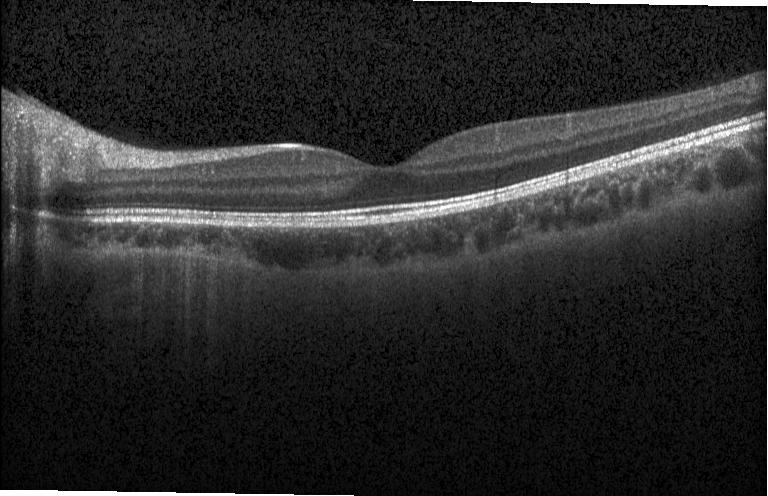

The scan shows no evidence of CNV, DME, or drusen.